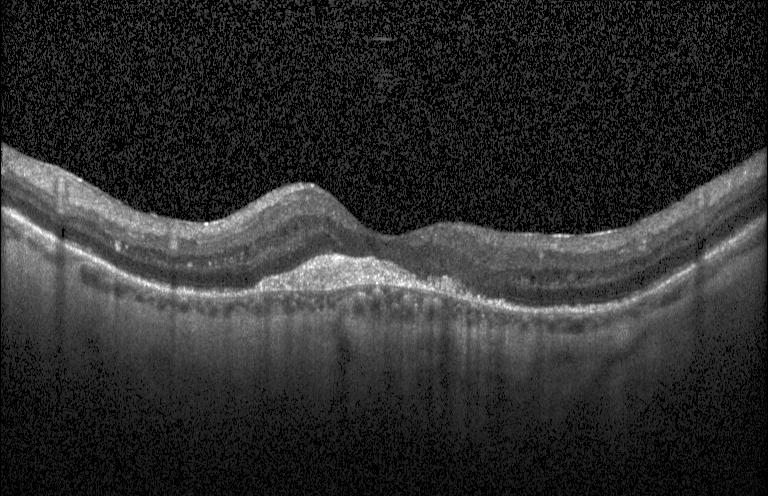
Dx: choroidal neovascularization.